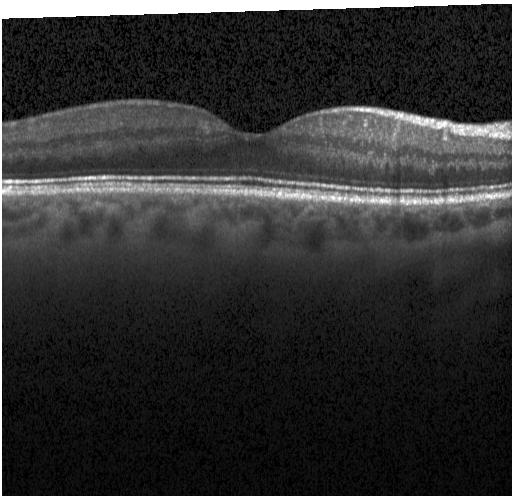

Retinal OCT B-scan — This B-scan demonstrates neither choroidal neovascularization, diabetic macular edema, nor drusen.